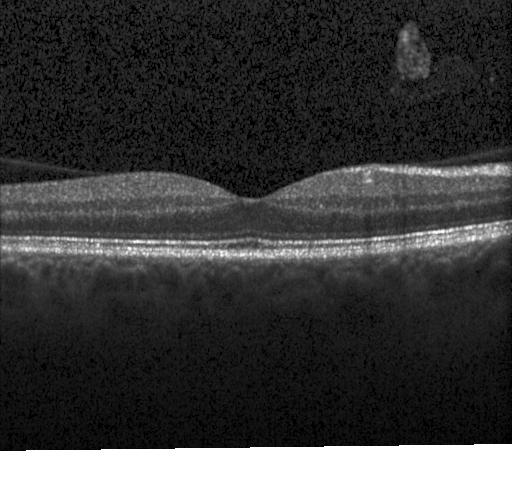
Retinal OCT cross-section. Centered on the fovea. Spectral-domain OCT. Heidelberg Spectralis OCT system
Dx: no choroidal neovascularization, diabetic macular edema, or drusen.